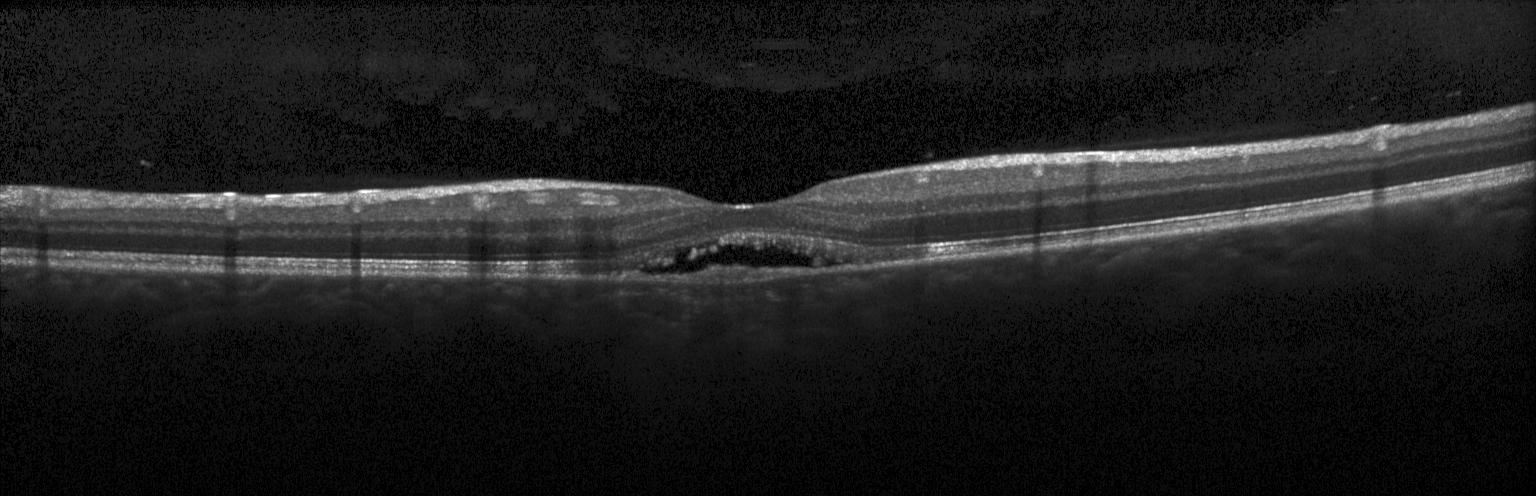
OCT B-scan showing a choroidal neovascular membrane.